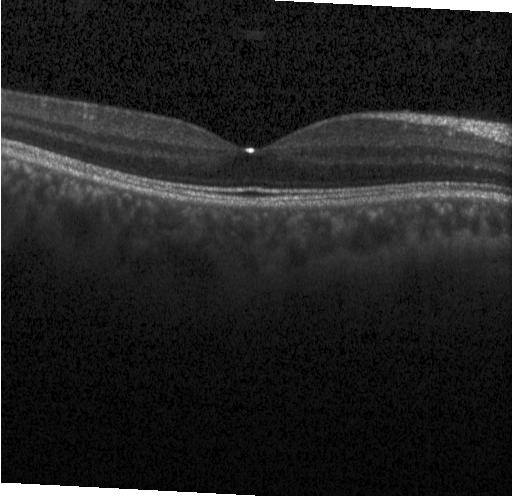
Impression: no choroidal neovascularization, no diabetic macular edema, and no drusen.